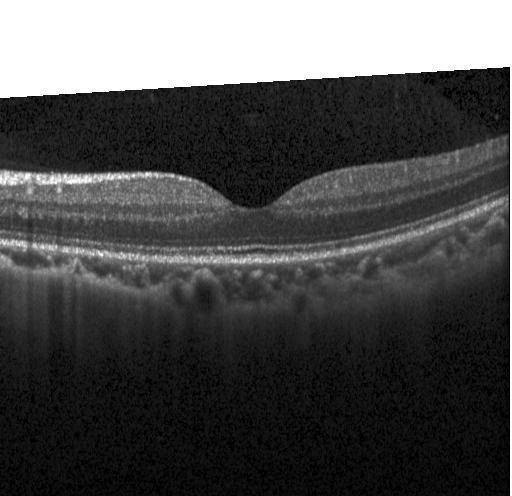 Macular OCT demonstrating no CNV, no DME, and no drusen.